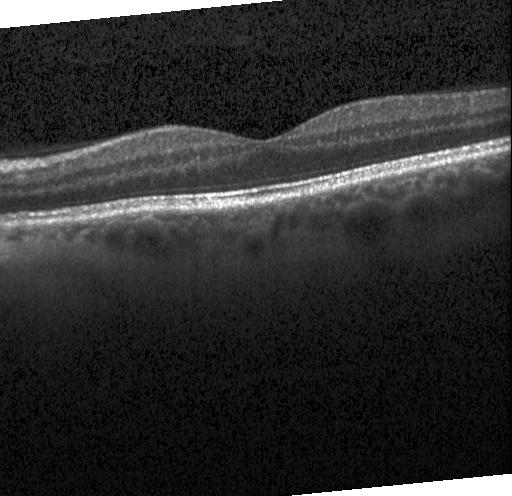
OCT line scan, SD-OCT.
Diagnosis: no CNV, no DME, and no drusen.